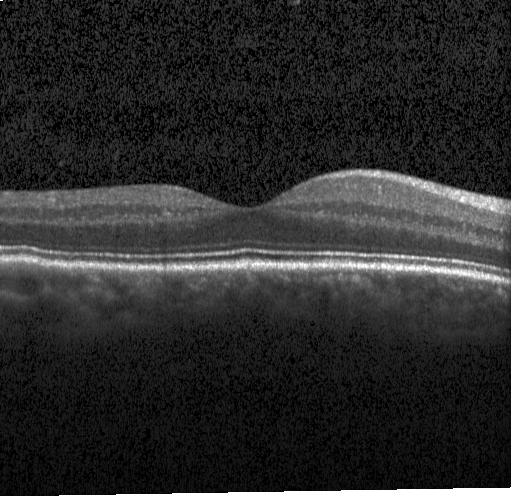
Optical coherence tomography B-scan.
Finding: neither choroidal neovascularization, diabetic macular edema, nor drusen.